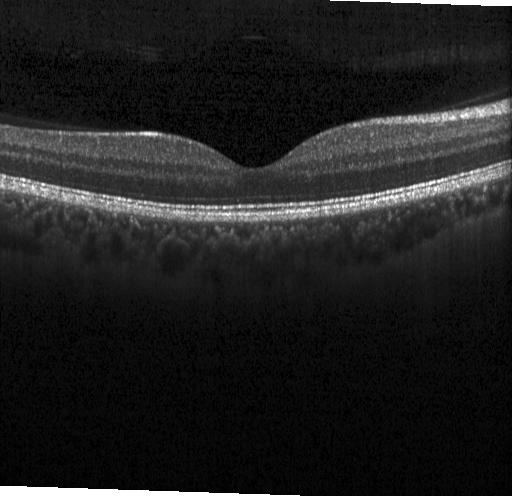

OCT scan showing no evidence of choroidal neovascularization, diabetic macular edema, or drusen.